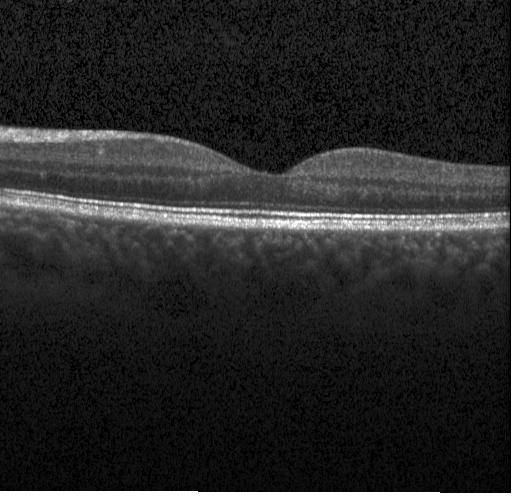 SD-OCT. Retinal OCT cross-section. Finding: no evidence of choroidal neovascularization, diabetic macular edema, or drusen.